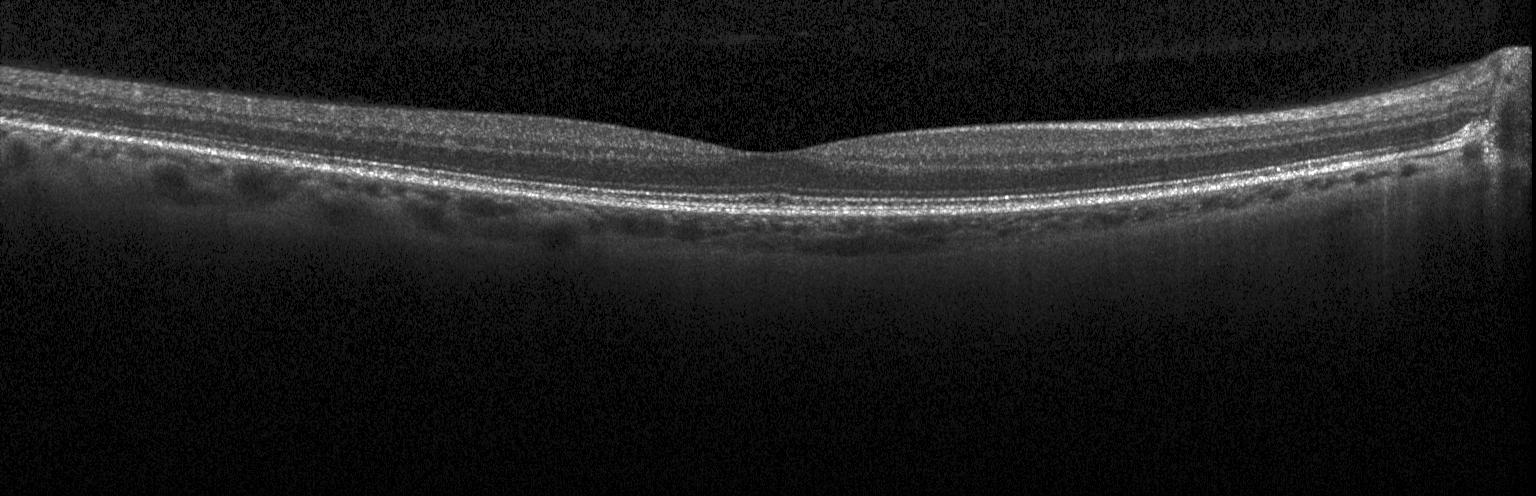
Horizontal scan through the fovea · OCT line scan
The scan shows no evidence of choroidal neovascularization, diabetic macular edema, or drusen.